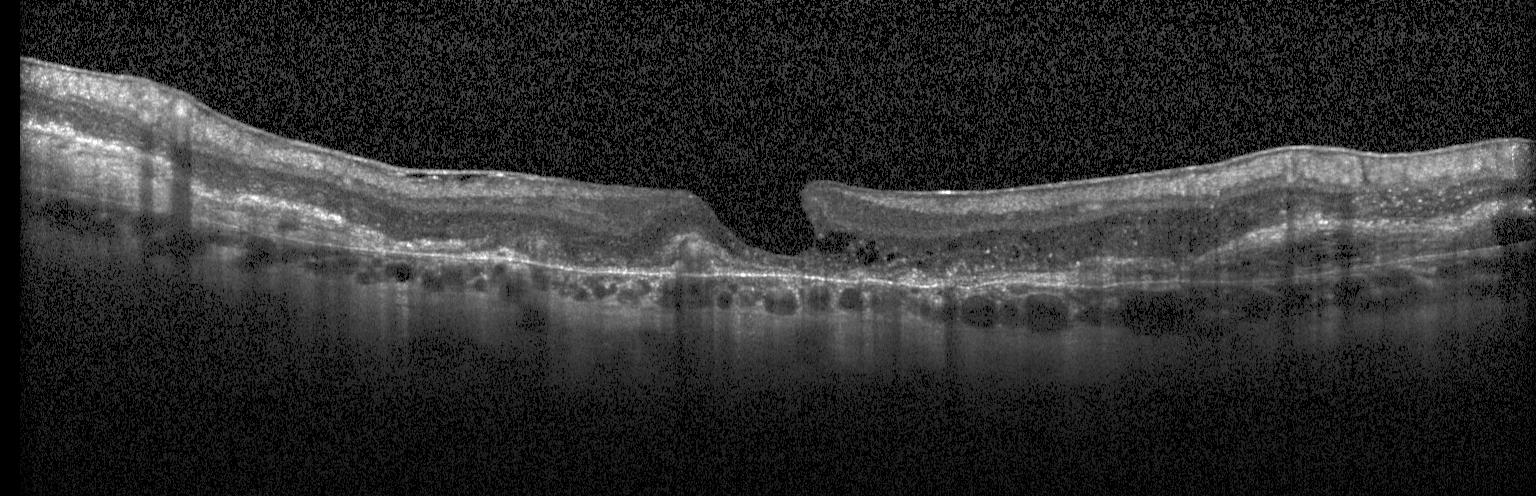

Heidelberg Spectralis OCT system; centered on the fovea; OCT line scan
Finding: CNV.